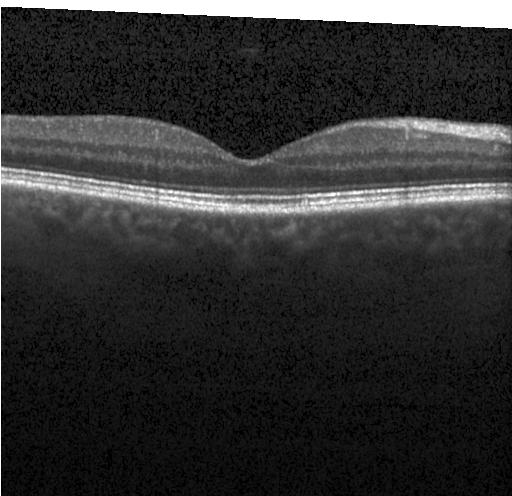 OCT B-scan showing neither choroidal neovascularization, diabetic macular edema, nor drusen.